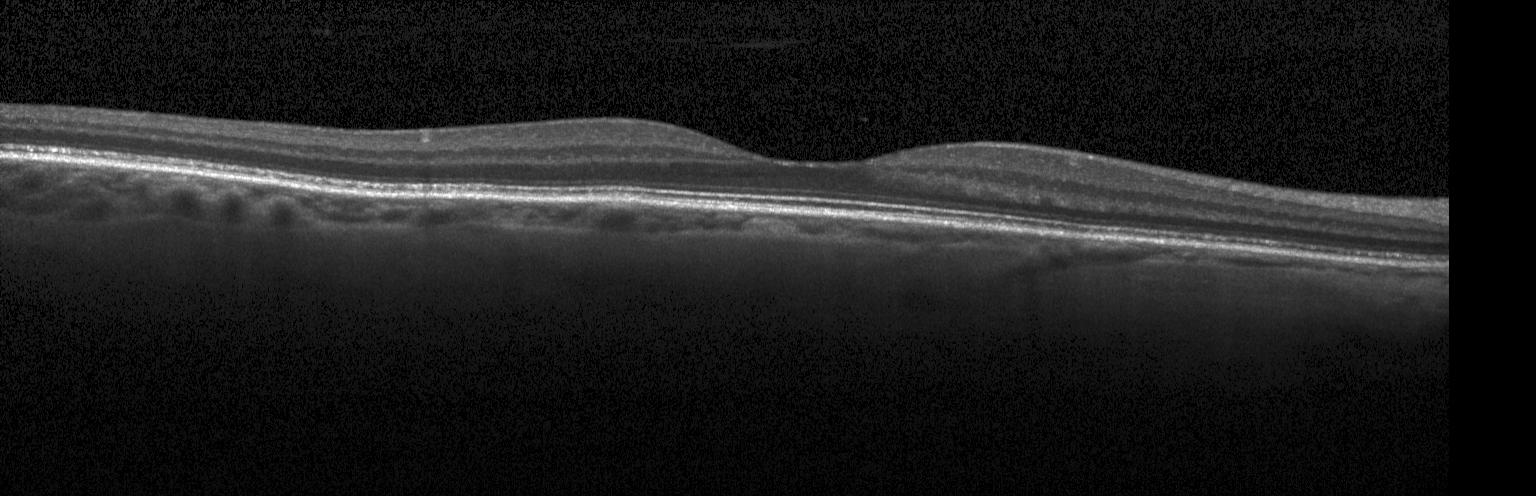
Macular OCT: no evidence of choroidal neovascularization, diabetic macular edema, or drusen.